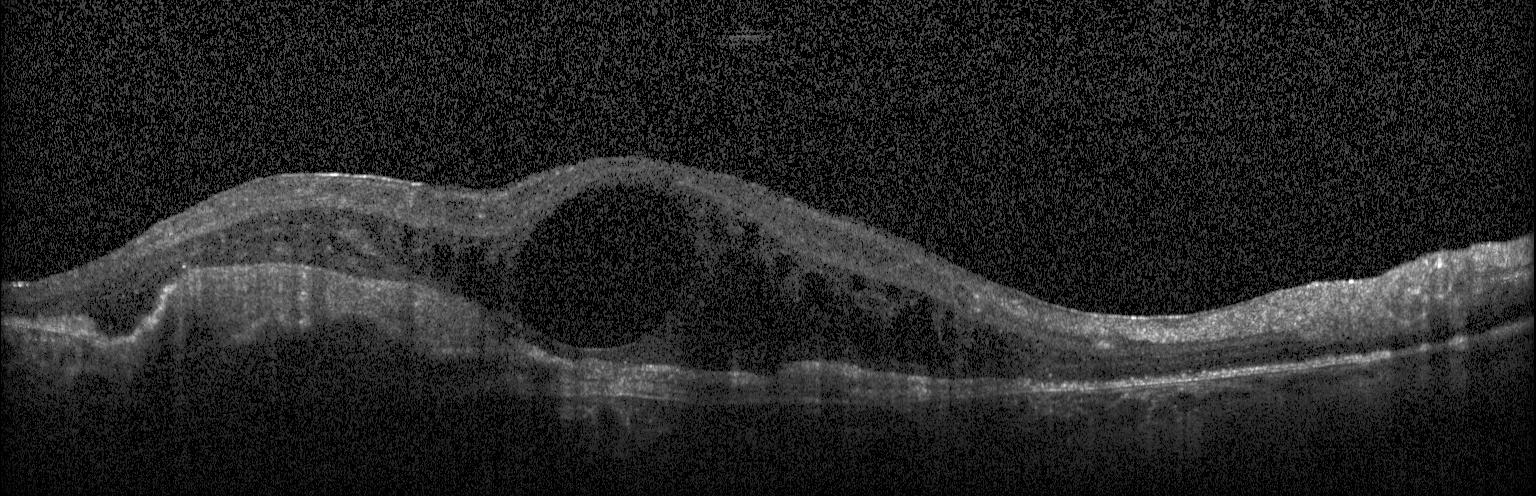

OCT B-scan
This B-scan demonstrates choroidal neovascularization (CNV).